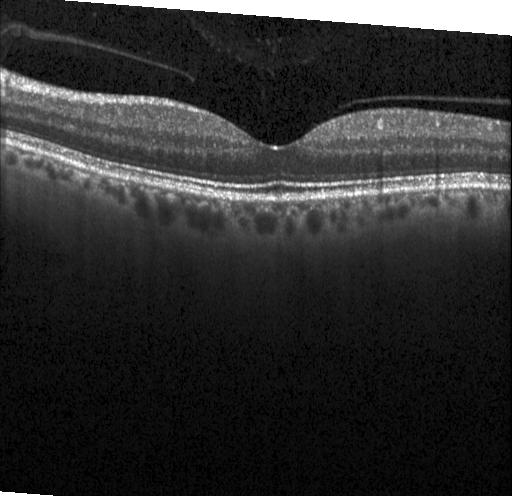
Dx: no CNV, no DME, and no drusen.